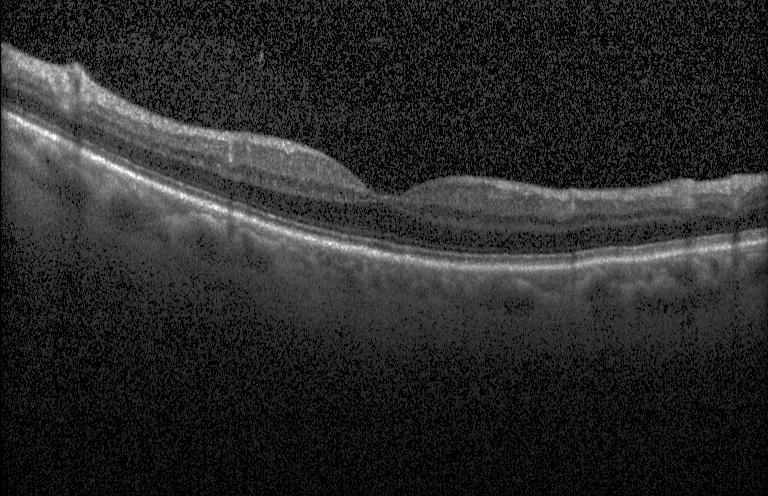
OCT scan showing neither CNV, DME, nor drusen.